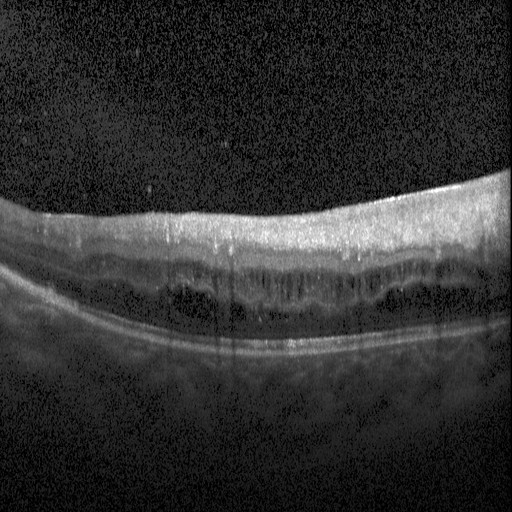 Retinal OCT B-scan, Heidelberg Spectralis OCT system, horizontal scan through the fovea. Impression: diabetic macular edema (DME).